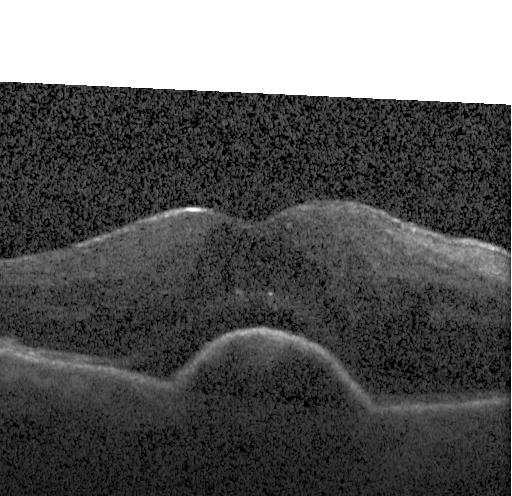
OCT finding: a choroidal neovascular membrane.